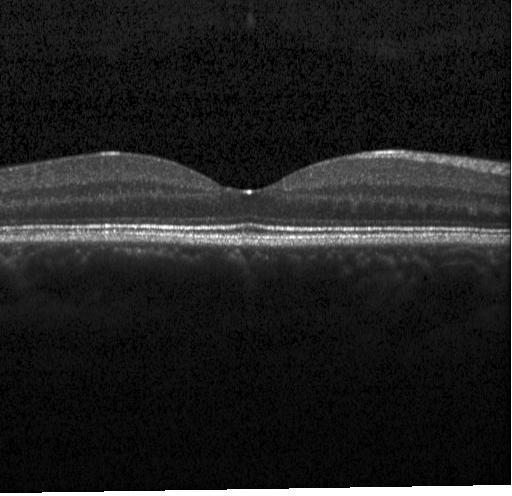
SD-OCT · OCT B-scan · instrument: Heidelberg Spectralis.
Dx: neither choroidal neovascularization, diabetic macular edema, nor drusen.